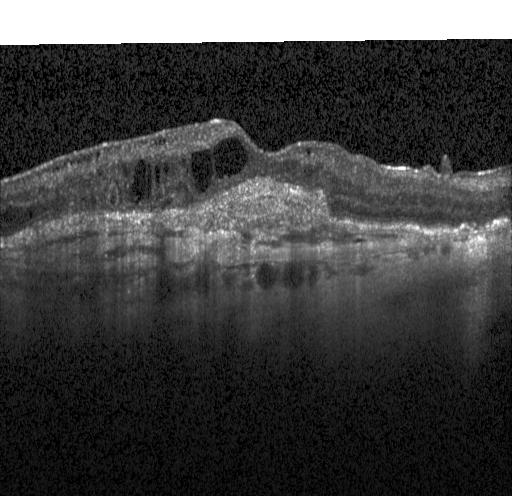
Retinal OCT cross-section.
CNV.